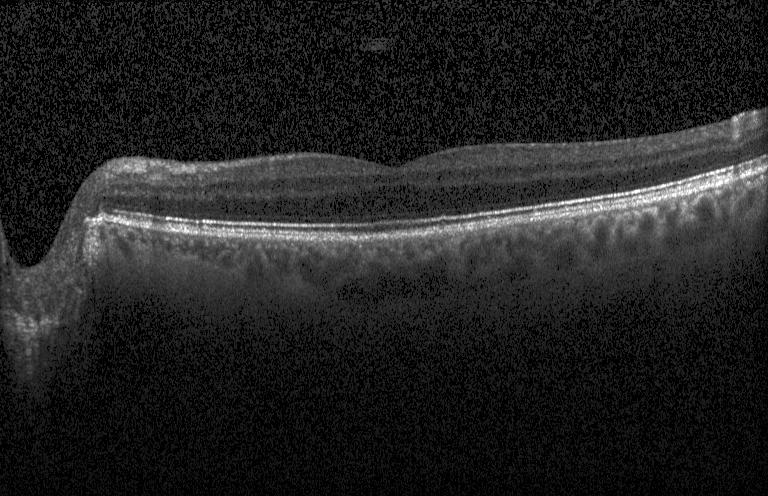

Impression: neither choroidal neovascularization, diabetic macular edema, nor drusen.